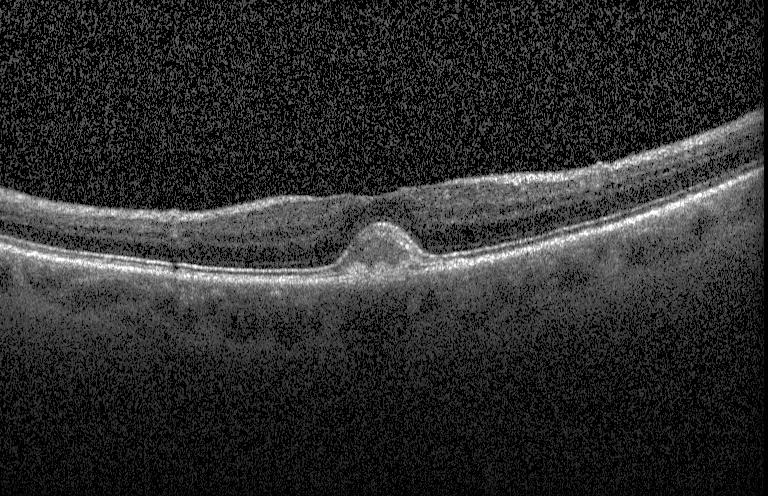

SD-OCT, instrument: Heidelberg Spectralis, horizontal scan through the fovea, OCT line scan
Diagnosis: a choroidal neovascular membrane.